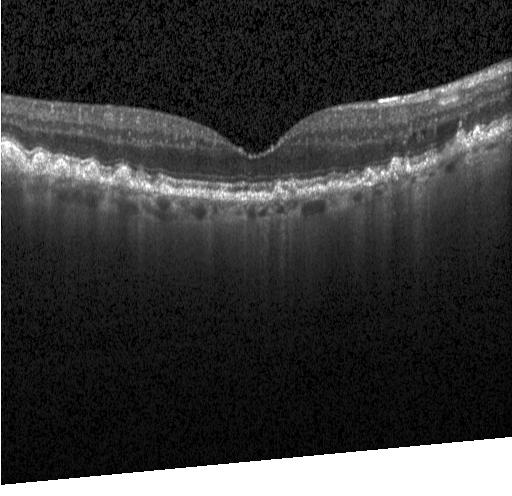
OCT finding: drusen.